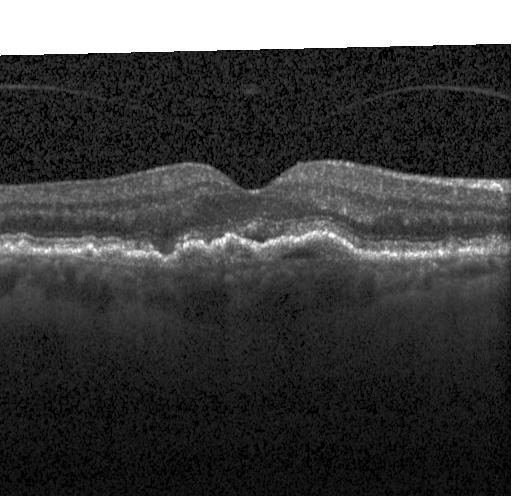

Retinal OCT B-scan; Heidelberg Spectralis OCT system — This B-scan demonstrates choroidal neovascularization (CNV).